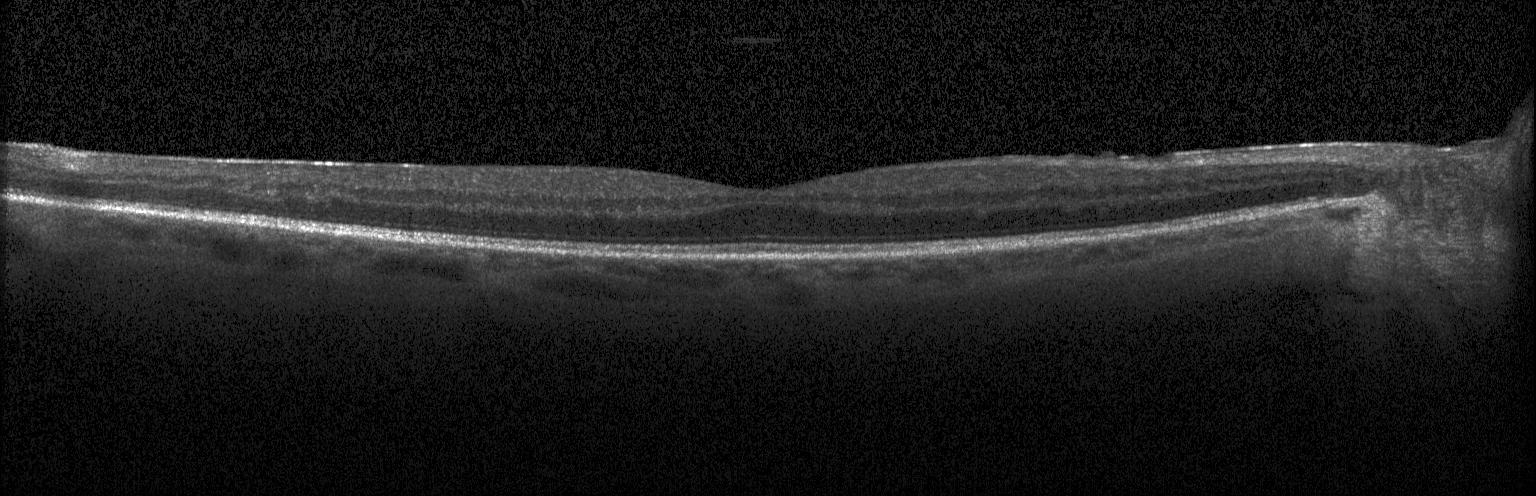

Optical coherence tomography scan.
Impression: neither choroidal neovascularization, diabetic macular edema, nor drusen.